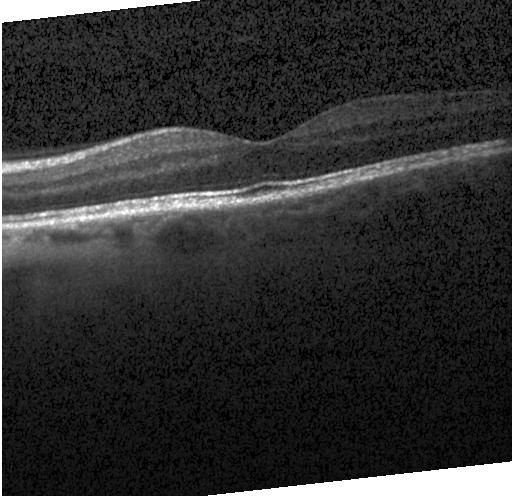
No choroidal neovascularization, no diabetic macular edema, and no drusen.